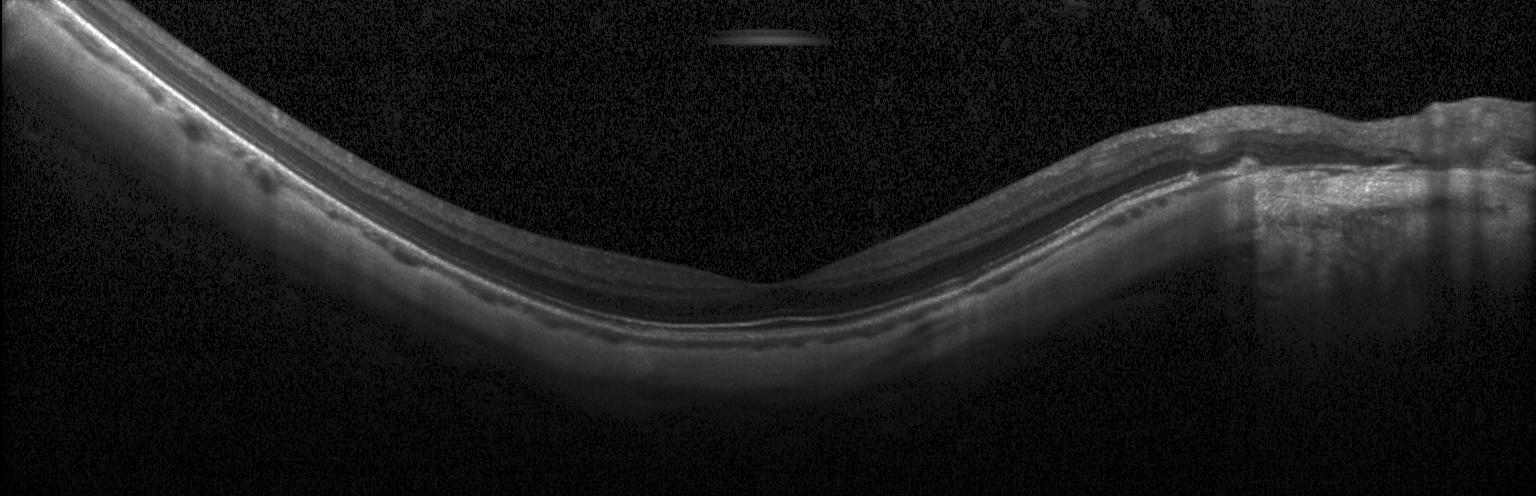
Finding: no CNV, DME, or drusen.